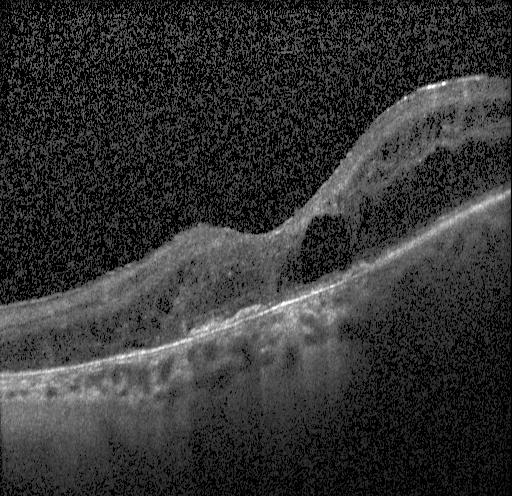
OCT scan showing CNV.